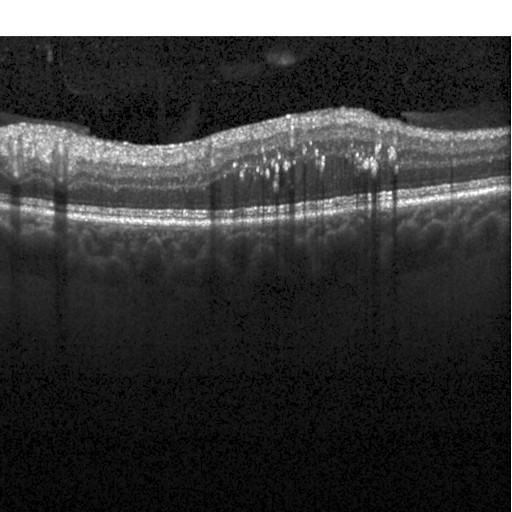

Optical coherence tomography scan. Fovea-centered. Finding: diabetic macular edema (DME).